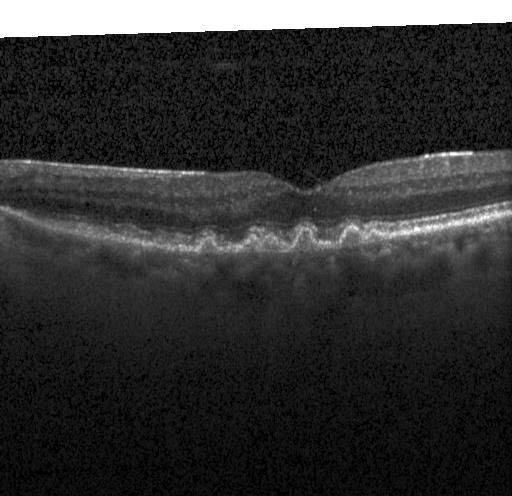

Through the macula · optical coherence tomography scan — Diagnosis: drusen.